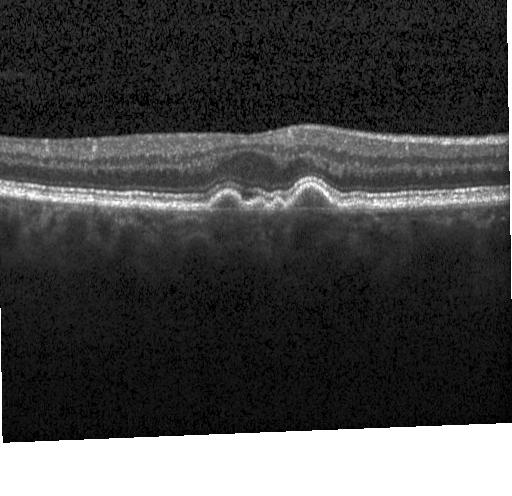
Retinal OCT B-scan.
Sub-RPE drusenoid deposits.